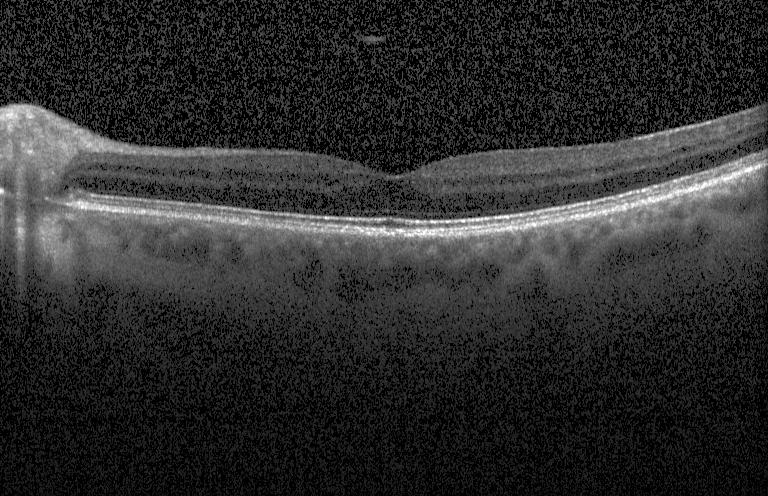

Retinal OCT cross-section showing no choroidal neovascularization, no diabetic macular edema, and no drusen.